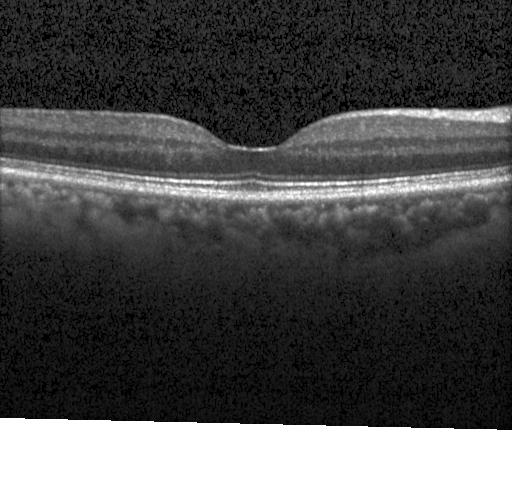

Optical coherence tomography scan · Heidelberg Spectralis OCT system. Finding: no CNV, no DME, and no drusen.